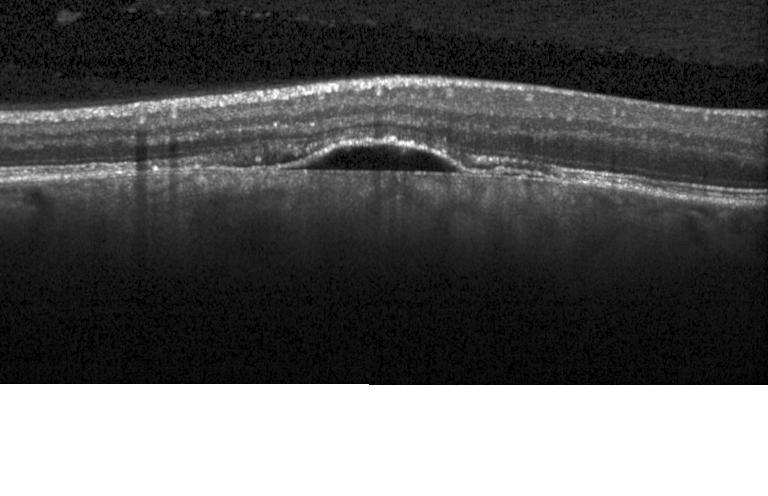 OCT line scan, spectral-domain OCT.
Assessment: a choroidal neovascular membrane.